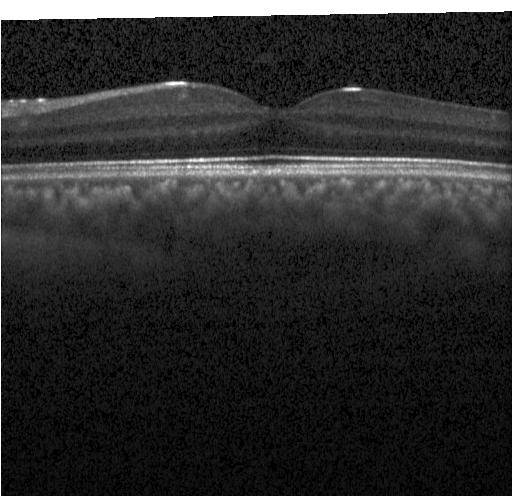
Retinal OCT B-scan · Heidelberg Spectralis
Finding: neither choroidal neovascularization, diabetic macular edema, nor drusen.